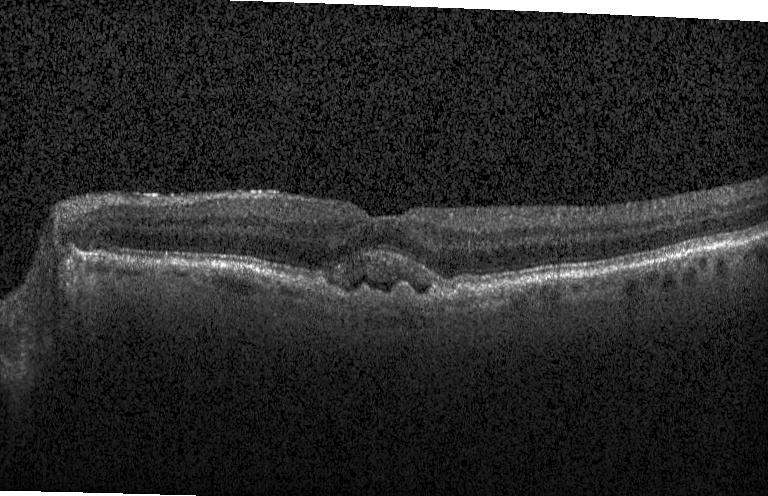
Retinal OCT B-scan, centered on the fovea — OCT finding: a choroidal neovascular membrane.